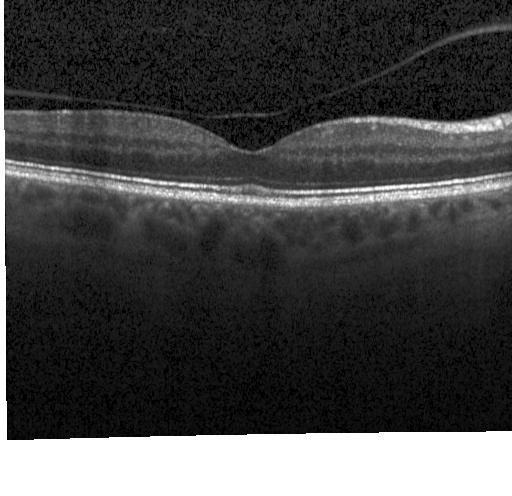

Macular OCT: no CNV, DME, or drusen.